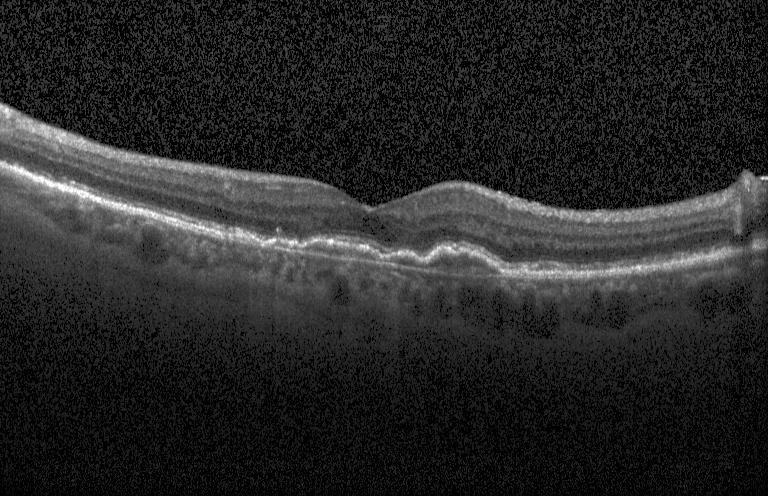
Spectral-domain optical coherence tomography; optical coherence tomography B-scan. Impression: CNV.